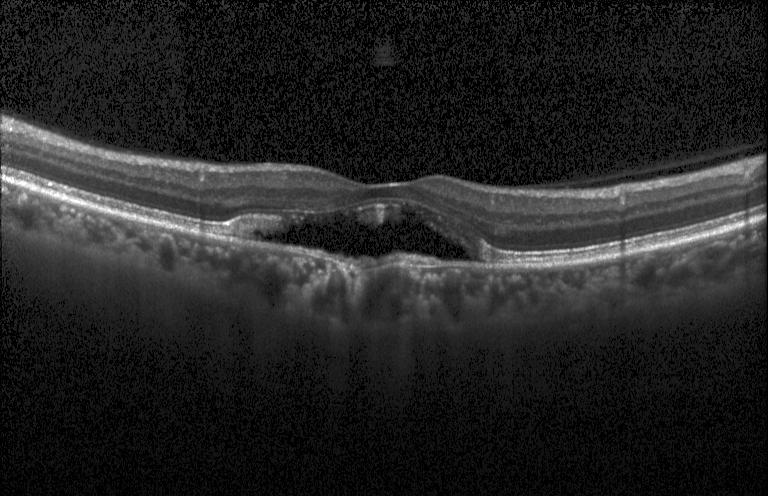
Diagnosis: choroidal neovascularization (CNV).